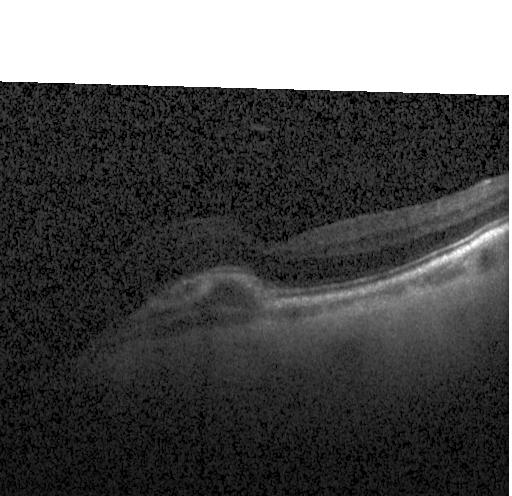 Heidelberg Spectralis. Spectral-domain optical coherence tomography. Fovea-centered. Optical coherence tomography B-scan — Impression: CNV.